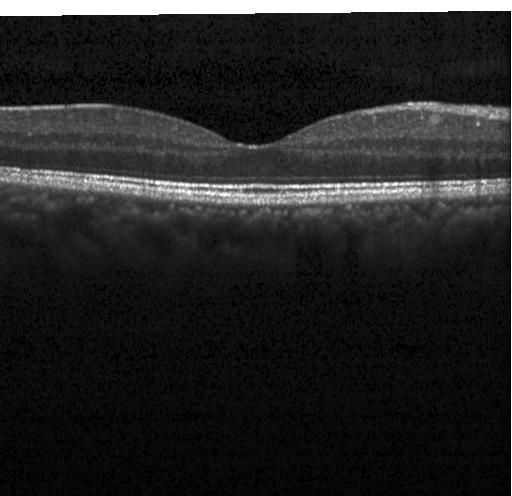 Spectral-domain OCT B-scan: no evidence of choroidal neovascularization, diabetic macular edema, or drusen.